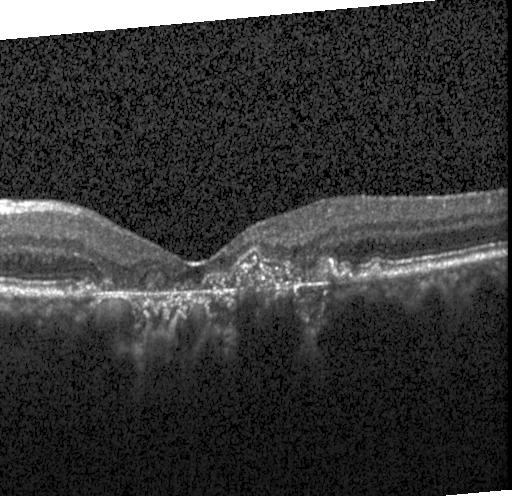 Macular scan; retinal OCT B-scan; Heidelberg Spectralis OCT system
Finding: a choroidal neovascular membrane.